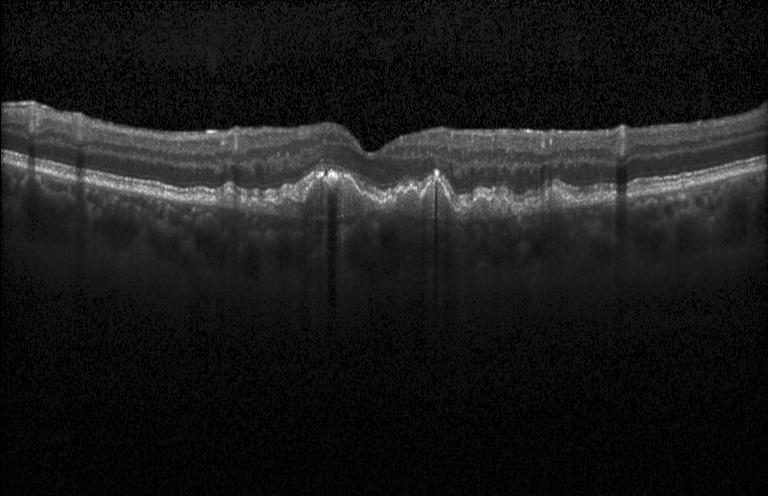 Optical coherence tomography scan · through the macula — Assessment: a choroidal neovascular membrane.